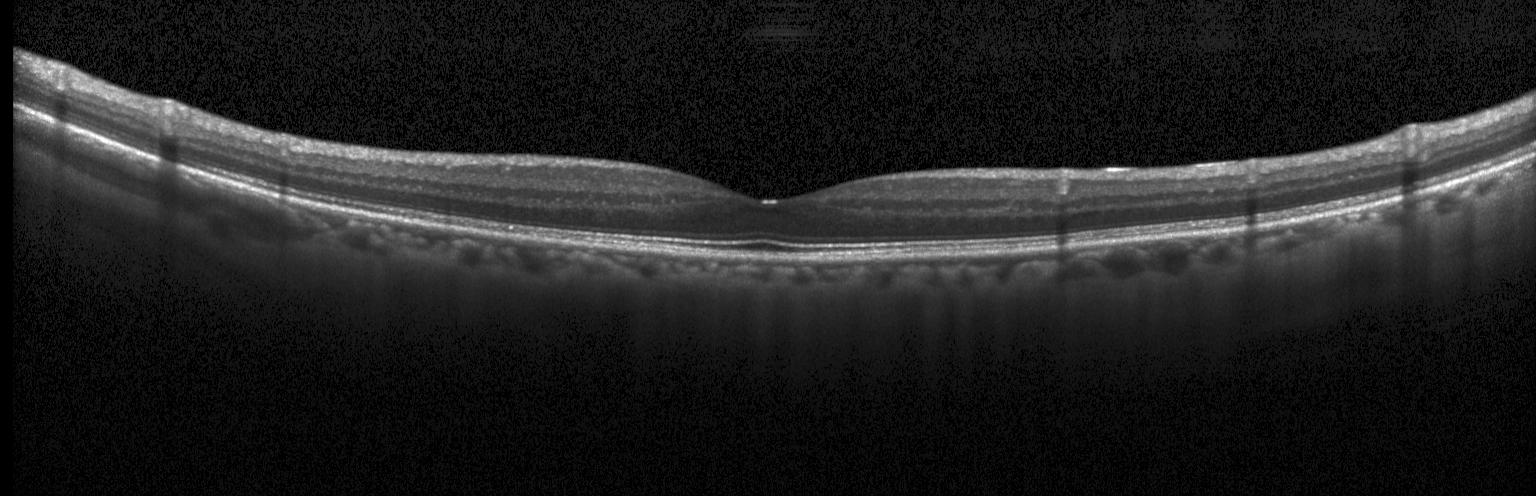
SD-OCT; retinal OCT B-scan; instrument: Heidelberg Spectralis. The scan shows no choroidal neovascularization, diabetic macular edema, or drusen.